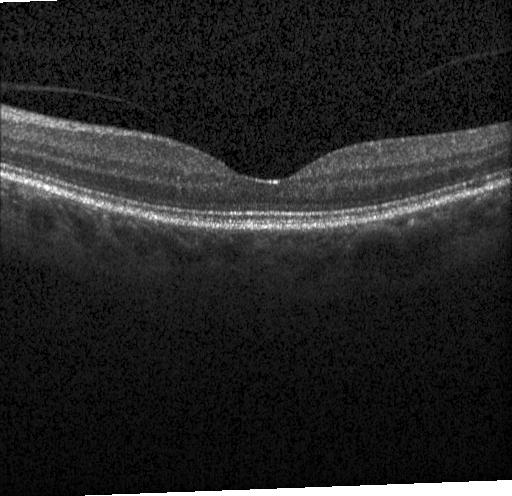

Fovea-centered; SD-OCT; optical coherence tomography B-scan; Heidelberg Spectralis
Neither choroidal neovascularization, diabetic macular edema, nor drusen.